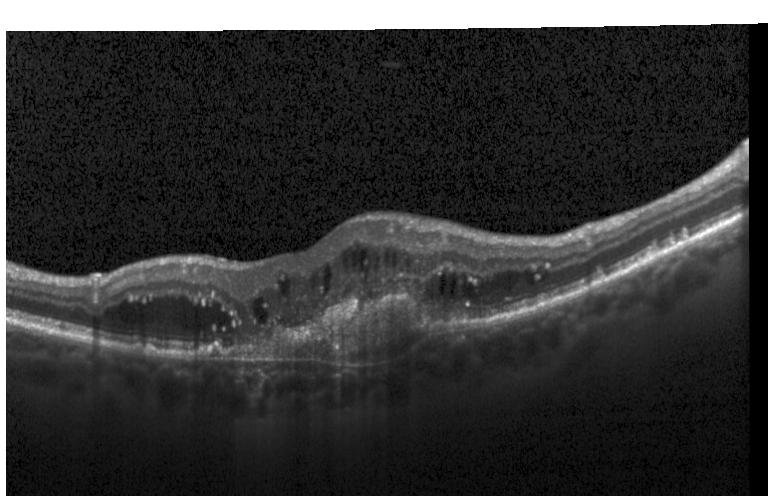 Impression: CNV.